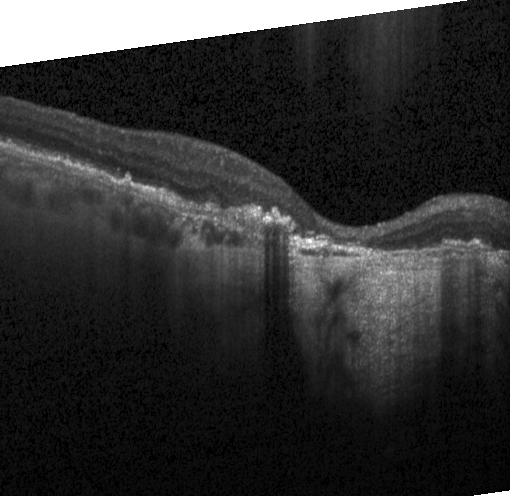
OCT line scan — Diagnosis: choroidal neovascularization (CNV).